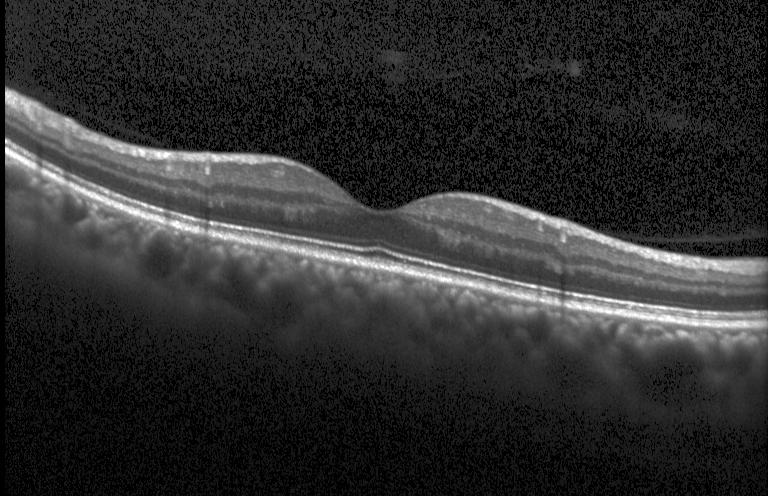
Finding: neither choroidal neovascularization, diabetic macular edema, nor drusen.